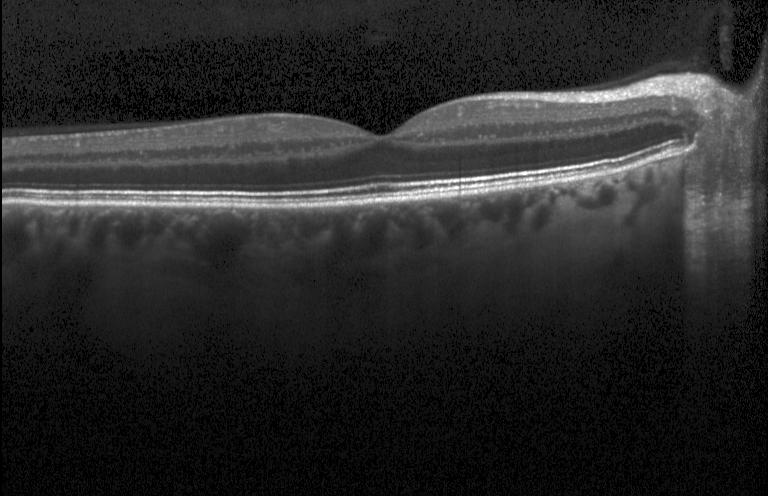
Macular scan, spectral-domain OCT, Heidelberg Spectralis OCT system, retinal OCT cross-section.
The scan shows neither choroidal neovascularization, diabetic macular edema, nor drusen.